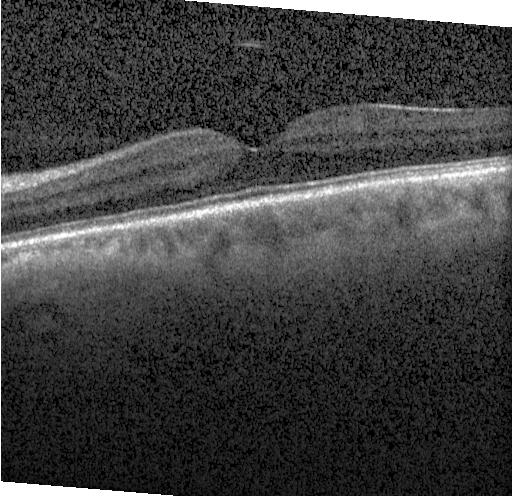
Fovea-centered · retinal OCT cross-section
The scan shows no evidence of choroidal neovascularization, diabetic macular edema, or drusen.